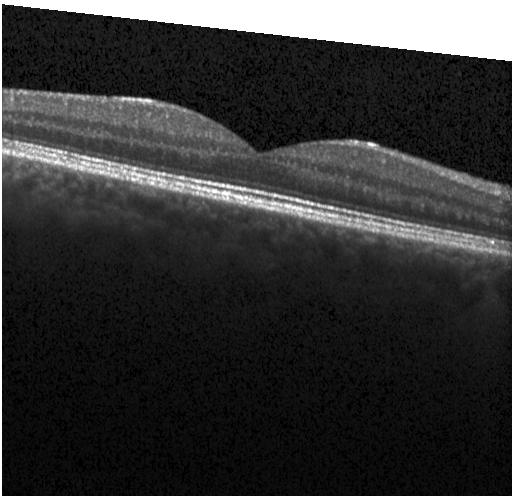

Through the macula · optical coherence tomography scan · acquired on a Heidelberg Spectralis
Neither choroidal neovascularization, diabetic macular edema, nor drusen.